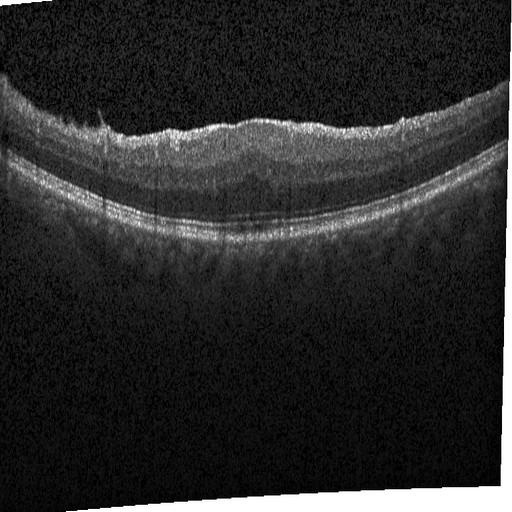

Diagnosis: diabetic macular edema.